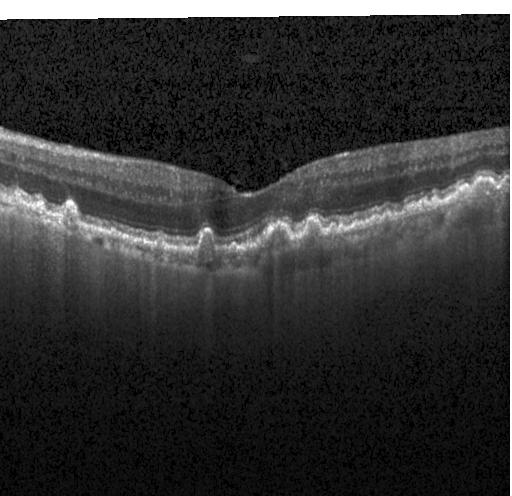 OCT line scan. Impression: sub-RPE drusenoid deposits.